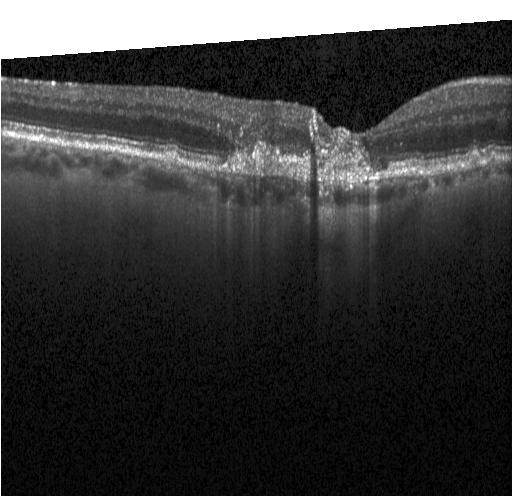

Macular OCT: a choroidal neovascular membrane.